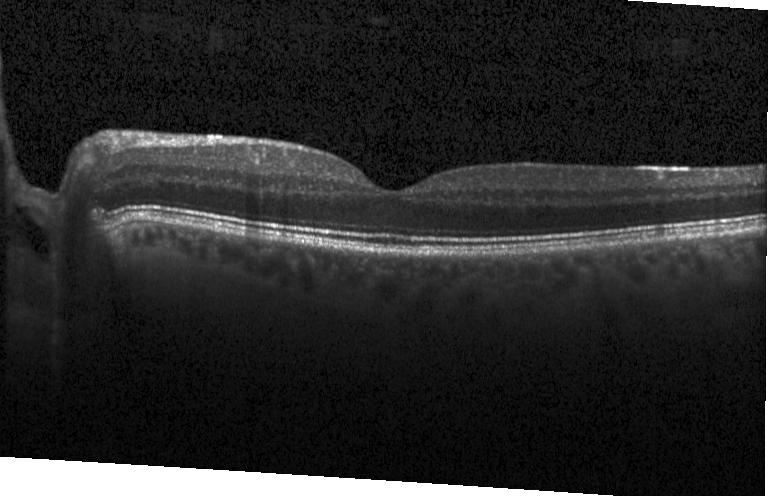

Impression: neither CNV, DME, nor drusen.